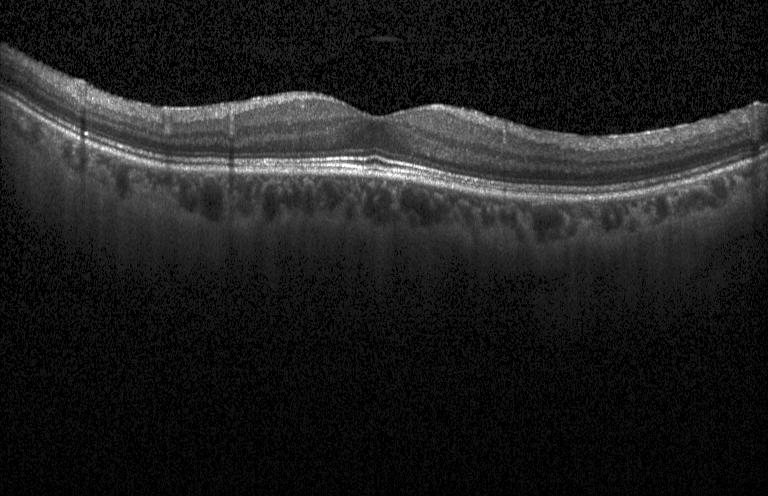

SD-OCT, OCT line scan, acquired on a Heidelberg Spectralis — This B-scan demonstrates neither CNV, DME, nor drusen.